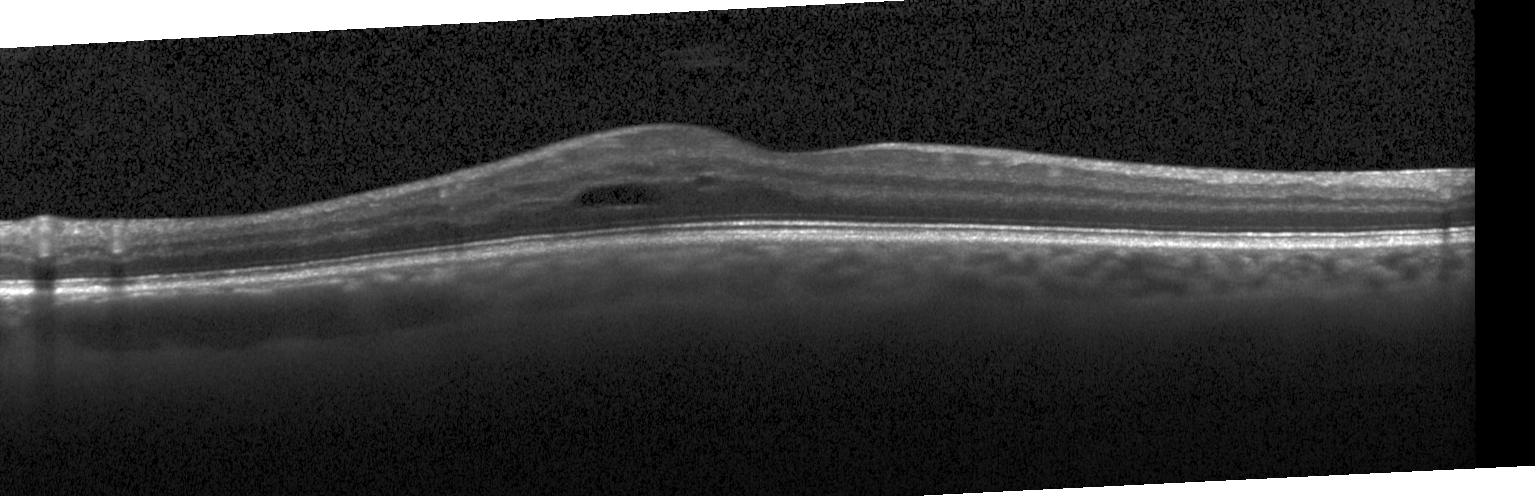
Spectral-domain OCT. Fovea-centered. OCT line scan. Heidelberg Spectralis — Impression: DME.